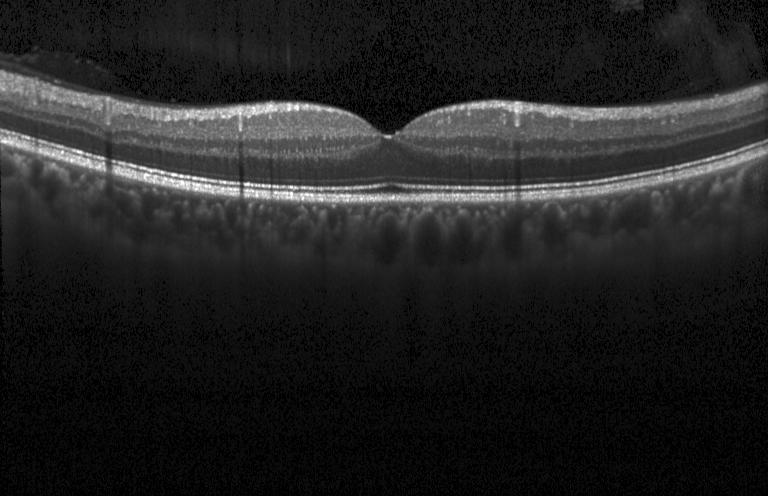
OCT B-scan.
Finding: no CNV, DME, or drusen.